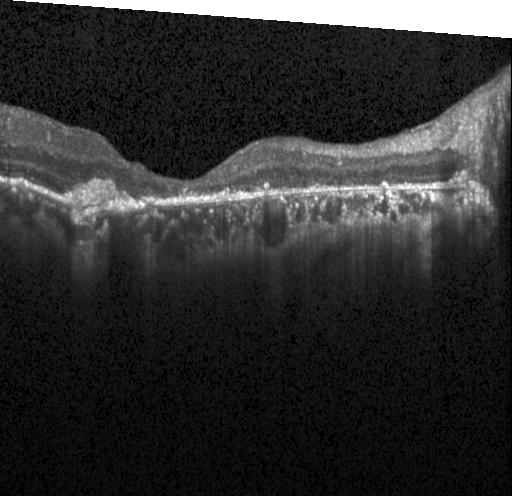 Diagnosis: a choroidal neovascular membrane.